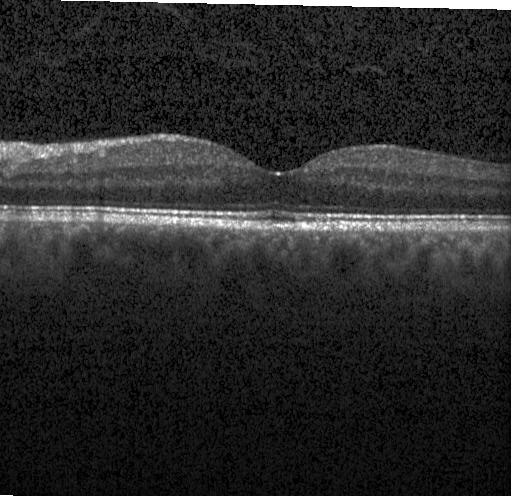

Assessment: neither choroidal neovascularization, diabetic macular edema, nor drusen.